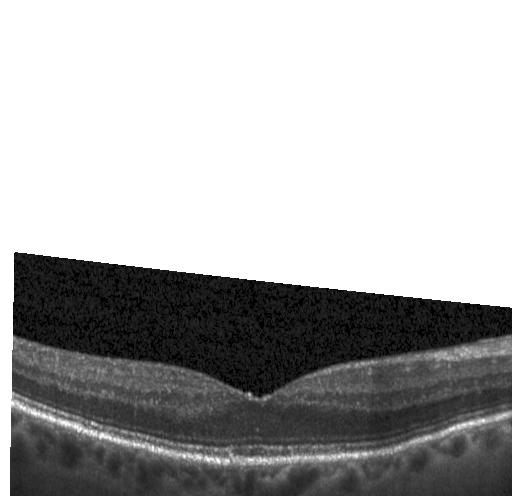 Retinal OCT B-scan · SD-OCT. Diagnosis: no evidence of CNV, DME, or drusen.